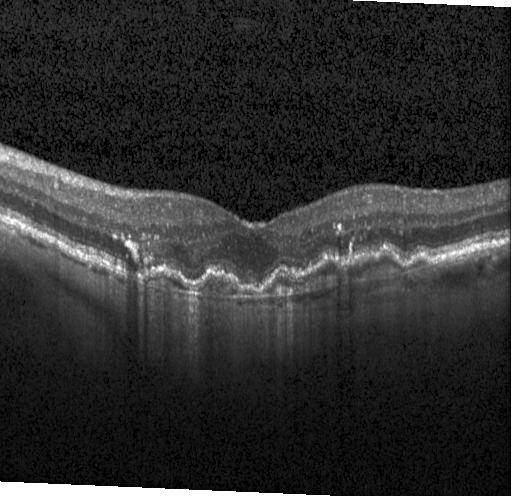

Optical coherence tomography B-scan · horizontal scan through the fovea.
Finding: choroidal neovascularization (CNV).